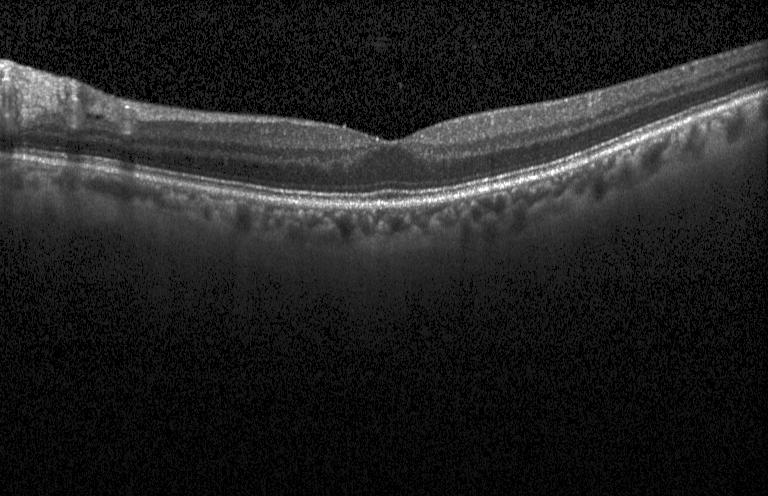

Diagnosis: no CNV, DME, or drusen.